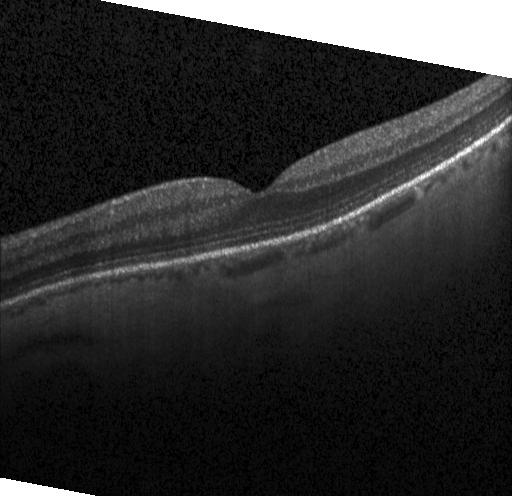

Centered on the fovea · spectral-domain optical coherence tomography · Heidelberg Spectralis · OCT B-scan — This B-scan demonstrates no choroidal neovascularization, diabetic macular edema, or drusen.